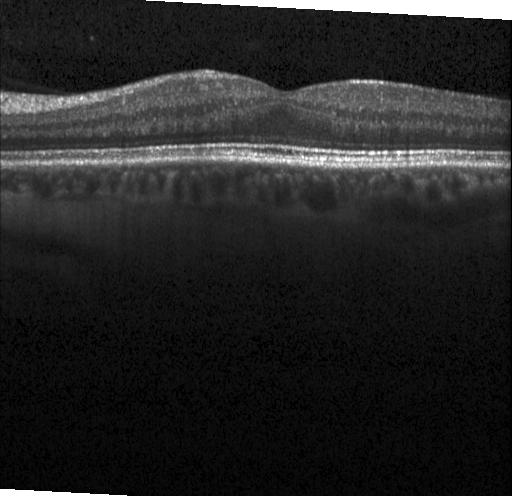

Horizontal scan through the fovea, retinal OCT cross-section, Heidelberg Spectralis, SD-OCT
OCT finding: no CNV, no DME, and no drusen.